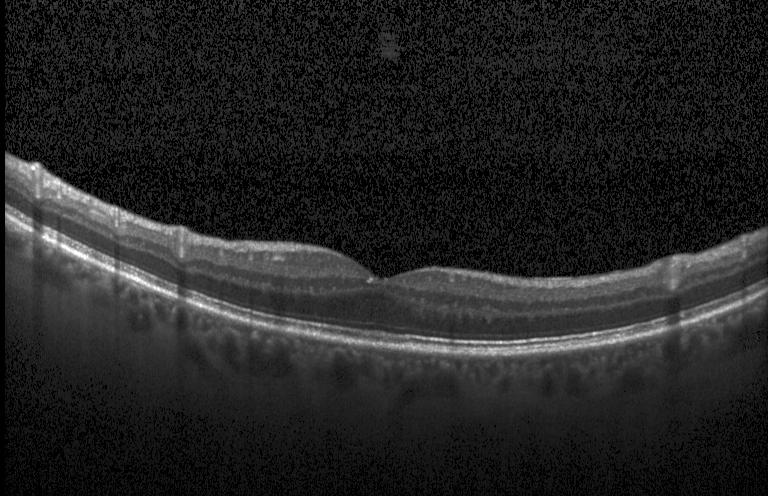
Retinal OCT B-scan
This B-scan demonstrates no evidence of choroidal neovascularization, diabetic macular edema, or drusen.